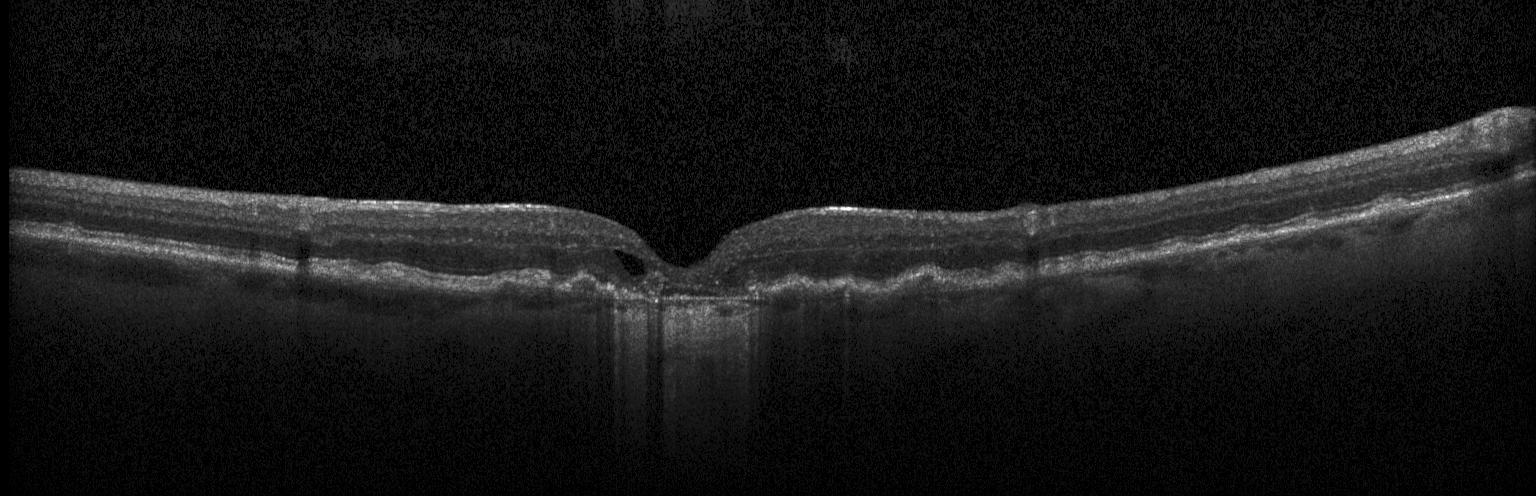
Choroidal neovascularization (CNV).